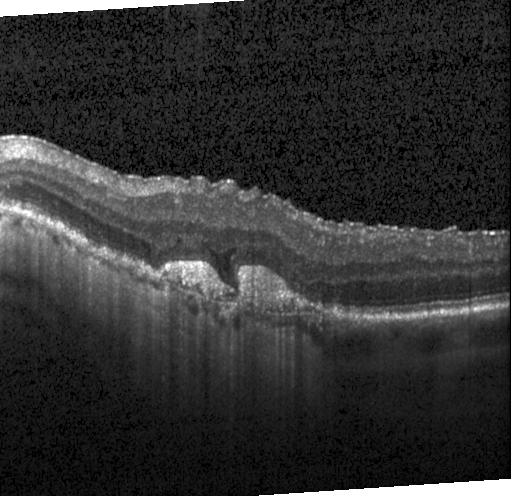
Finding: a choroidal neovascular membrane.